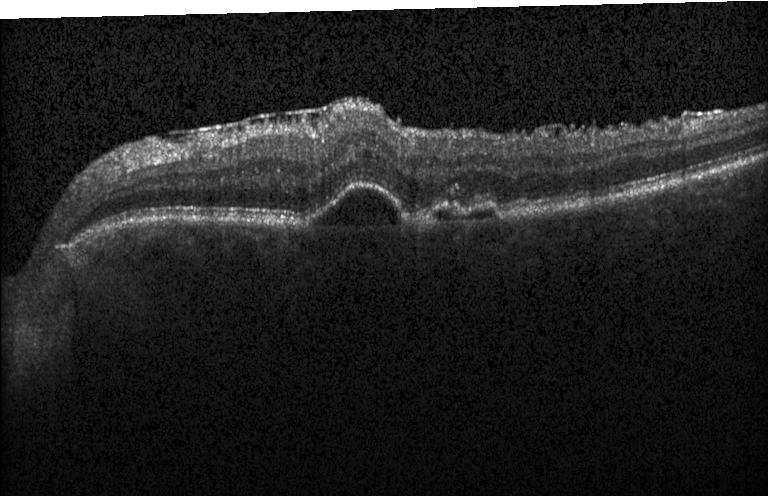 This B-scan demonstrates a choroidal neovascular membrane.